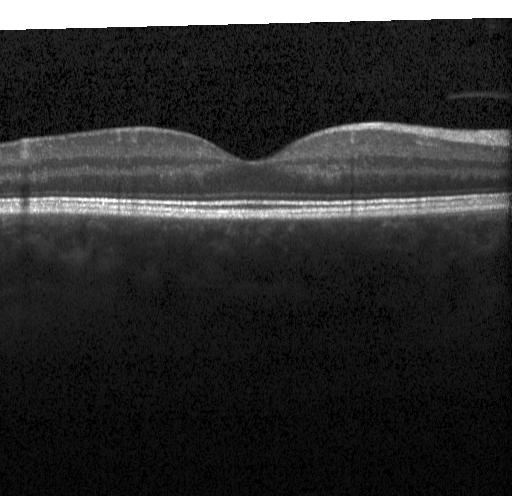
Assessment: neither choroidal neovascularization, diabetic macular edema, nor drusen.